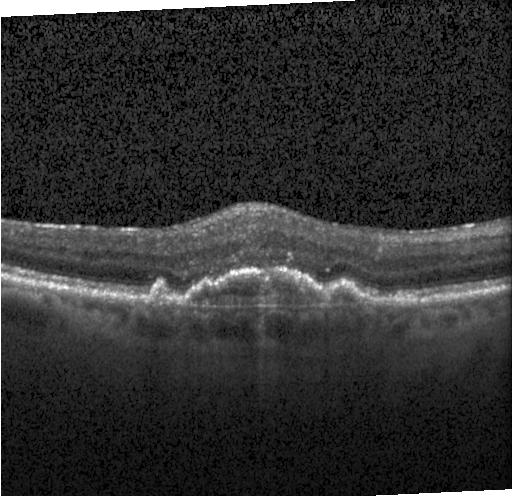
Retinal OCT B-scan, through the macula, spectral-domain OCT, Heidelberg Spectralis — Diagnosis: choroidal neovascularization (CNV).